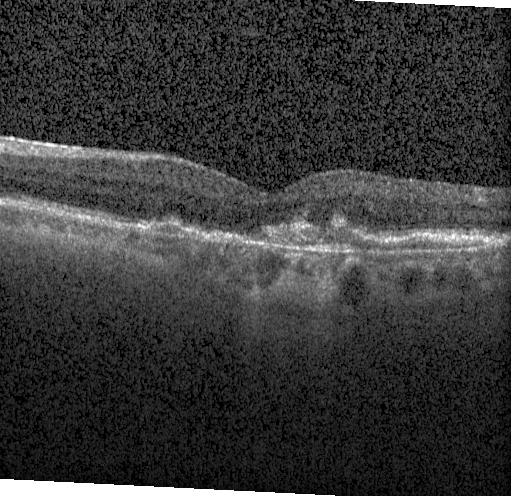
Spectral-domain OCT B-scan: a choroidal neovascular membrane.